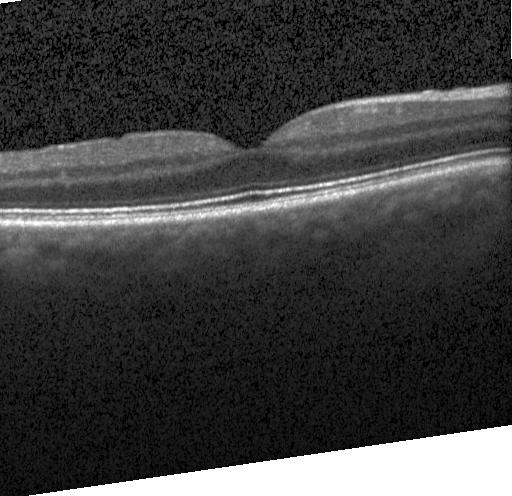 Horizontal scan through the fovea · instrument: Heidelberg Spectralis · retinal OCT B-scan.
Finding: neither CNV, DME, nor drusen.